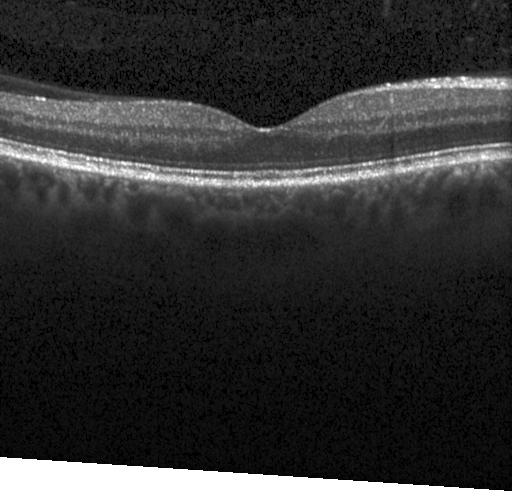

Instrument: Heidelberg Spectralis · optical coherence tomography B-scan · fovea-centered · spectral-domain optical coherence tomography.
Macular OCT: no choroidal neovascularization, no diabetic macular edema, and no drusen.